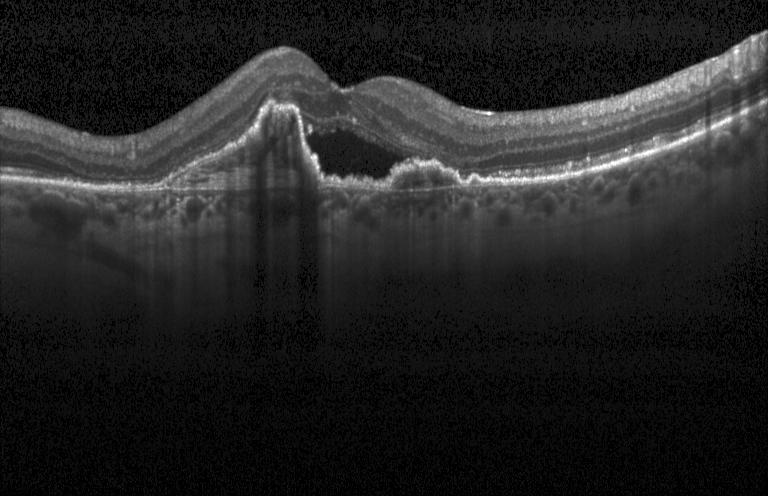 OCT finding: choroidal neovascularization.